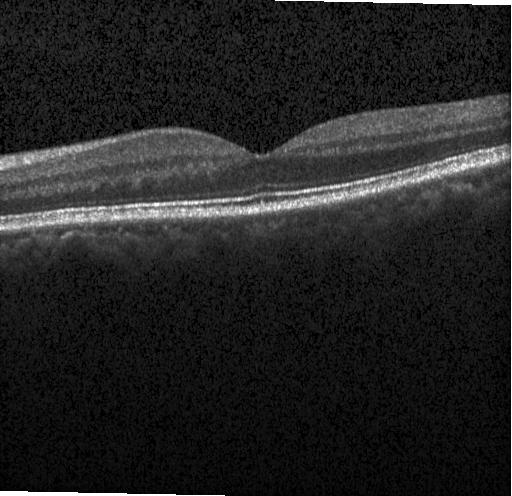 Spectral-domain optical coherence tomography. Optical coherence tomography B-scan.
This B-scan demonstrates no evidence of choroidal neovascularization, diabetic macular edema, or drusen.